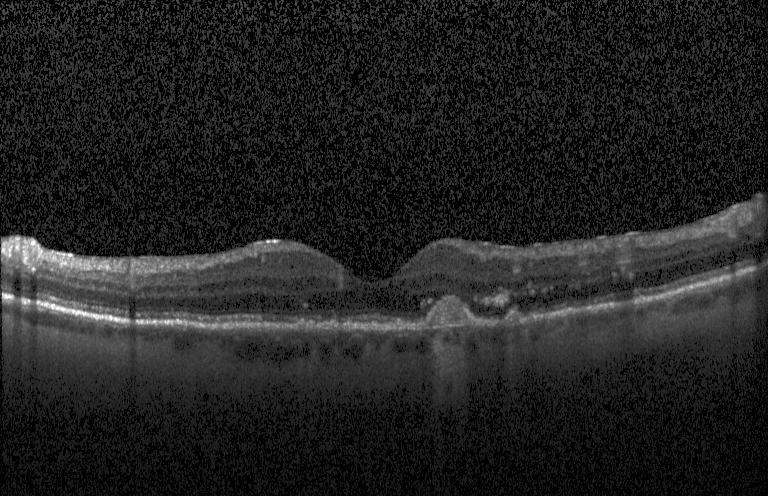 Through the macula. Optical coherence tomography B-scan. Heidelberg Spectralis
Drusen.